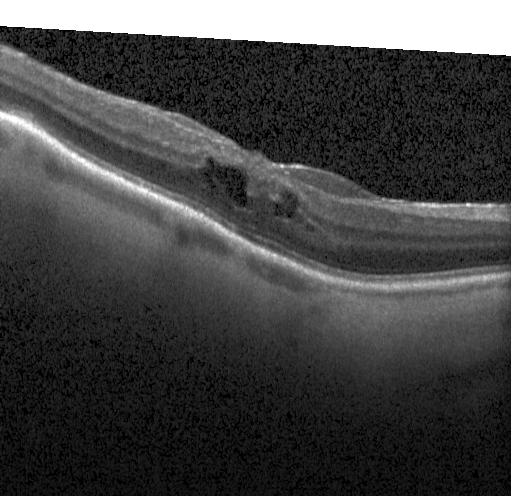
Diabetic macular edema (DME).